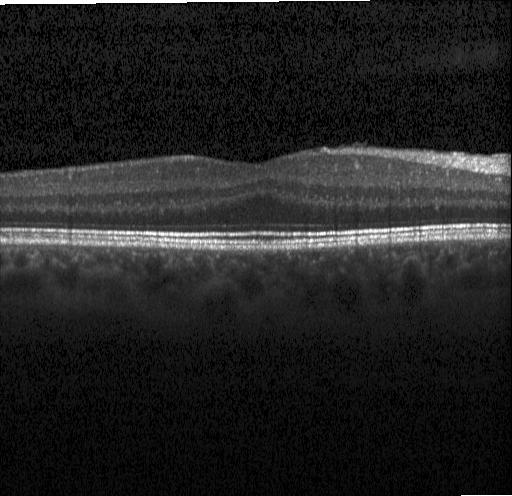 Retinal OCT cross-section.
Impression: no choroidal neovascularization, diabetic macular edema, or drusen.